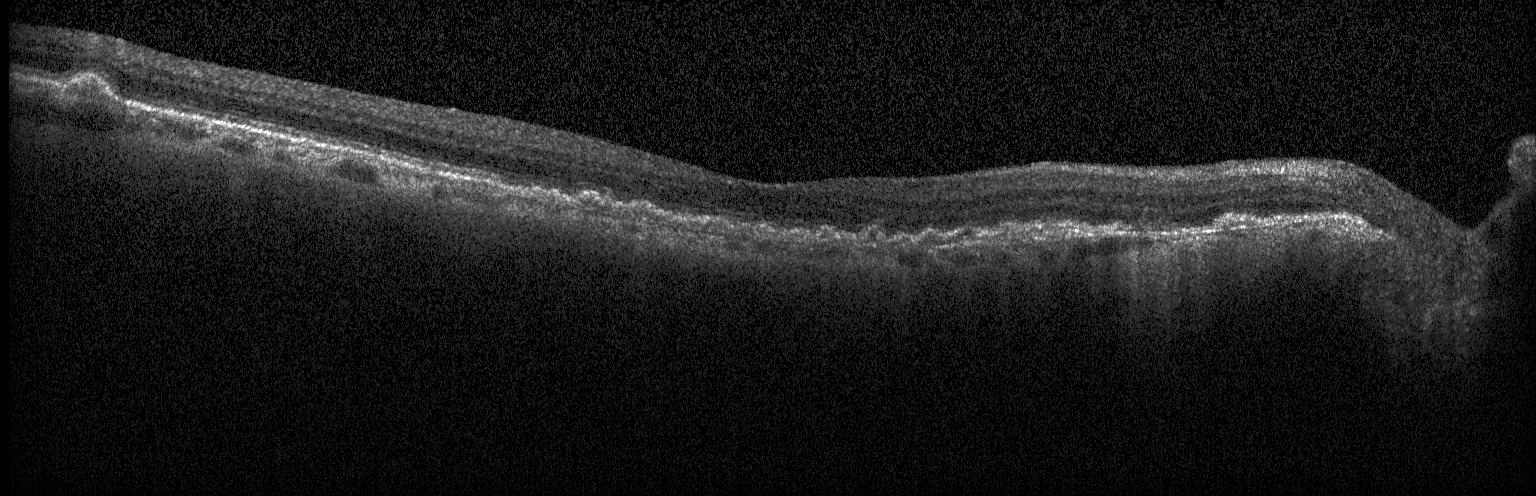 OCT finding: a choroidal neovascular membrane.